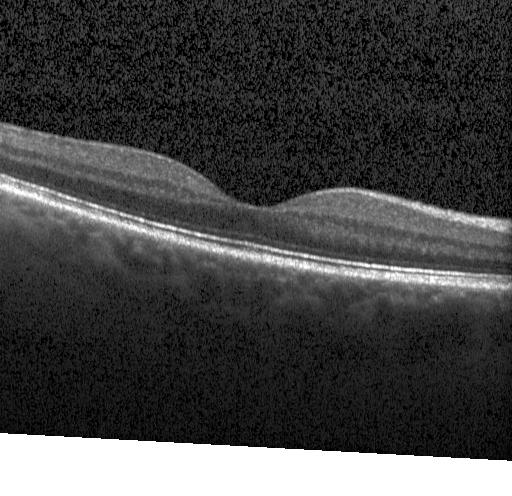 Macular OCT: no CNV, DME, or drusen.